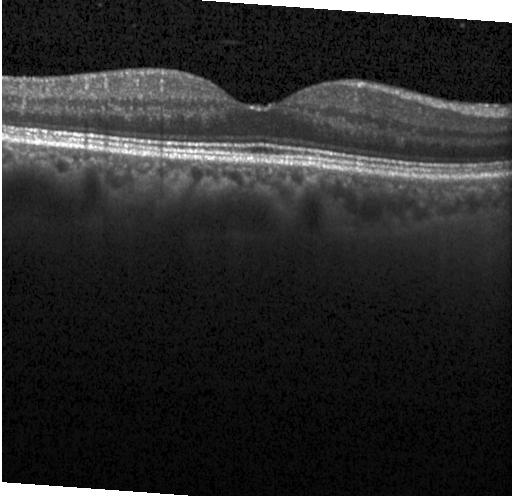

OCT B-scan. OCT finding: no choroidal neovascularization, diabetic macular edema, or drusen.